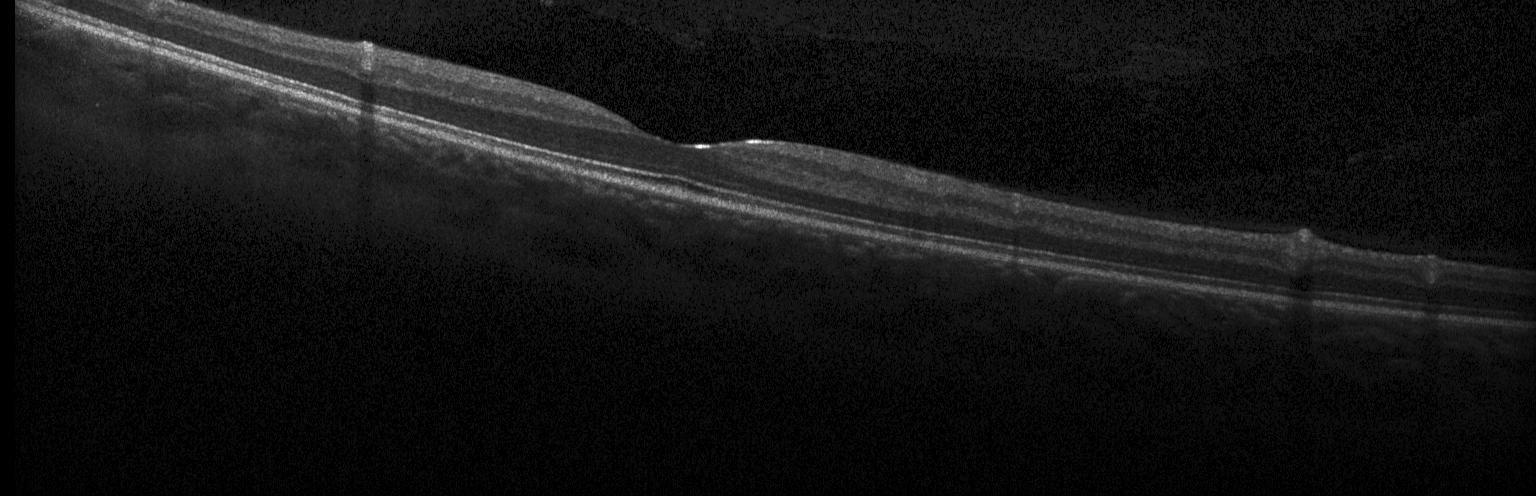
Fovea-centered; acquired on a Heidelberg Spectralis; spectral-domain optical coherence tomography; OCT B-scan.
Dx: neither choroidal neovascularization, diabetic macular edema, nor drusen.